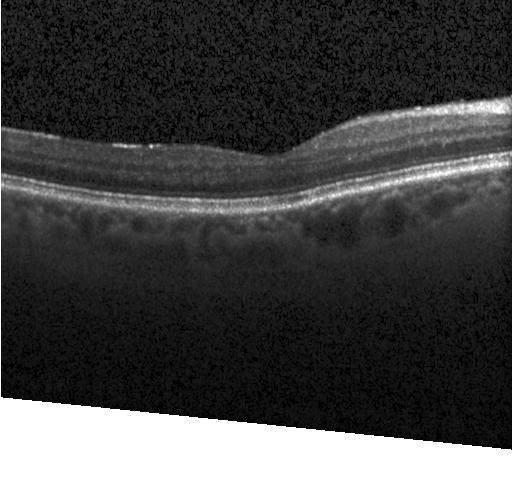

Macular OCT: no choroidal neovascularization, diabetic macular edema, or drusen.